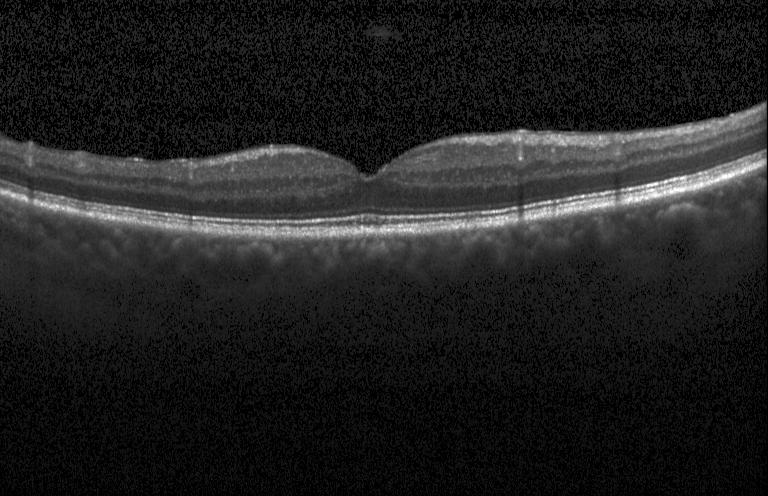

Acquired on a Heidelberg Spectralis. Optical coherence tomography B-scan. Neither choroidal neovascularization, diabetic macular edema, nor drusen.